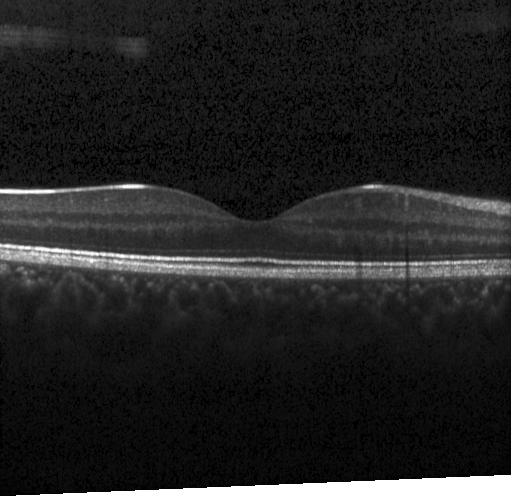 Centered on the fovea · spectral-domain OCT · Heidelberg Spectralis · OCT line scan.
Diagnosis: no choroidal neovascularization, no diabetic macular edema, and no drusen.